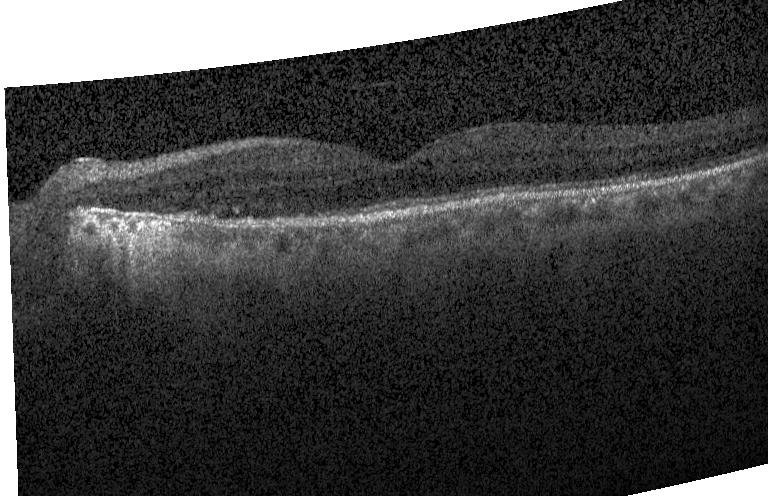

Retinal OCT B-scan, spectral-domain OCT, Heidelberg Spectralis, macular scan — The scan shows no choroidal neovascularization, no diabetic macular edema, and no drusen.